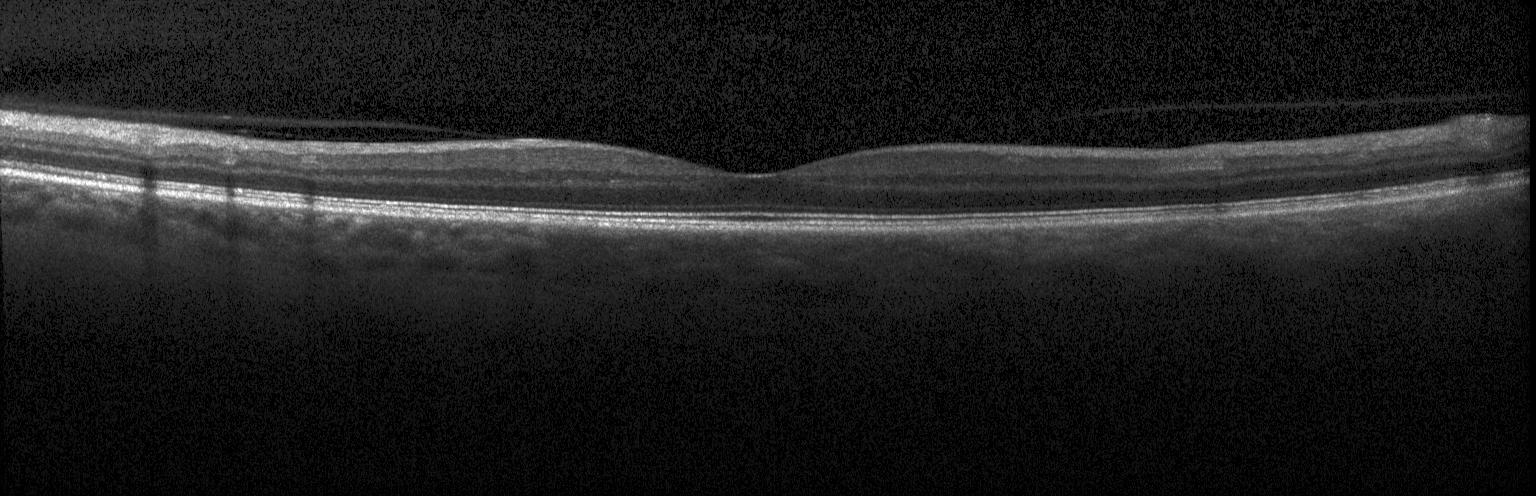 Retinal OCT B-scan. Heidelberg Spectralis OCT system. SD-OCT.
Diagnosis: neither choroidal neovascularization, diabetic macular edema, nor drusen.